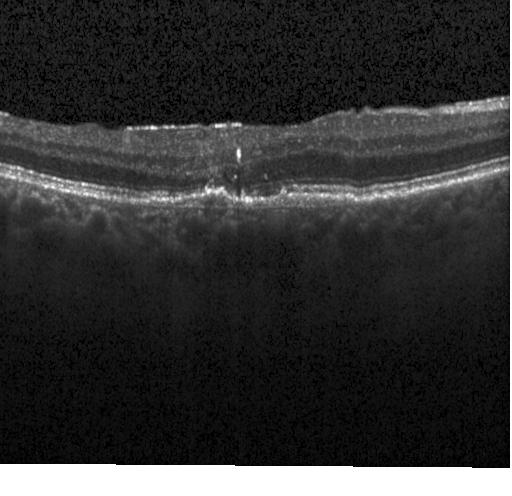
Diagnosis: choroidal neovascularization.